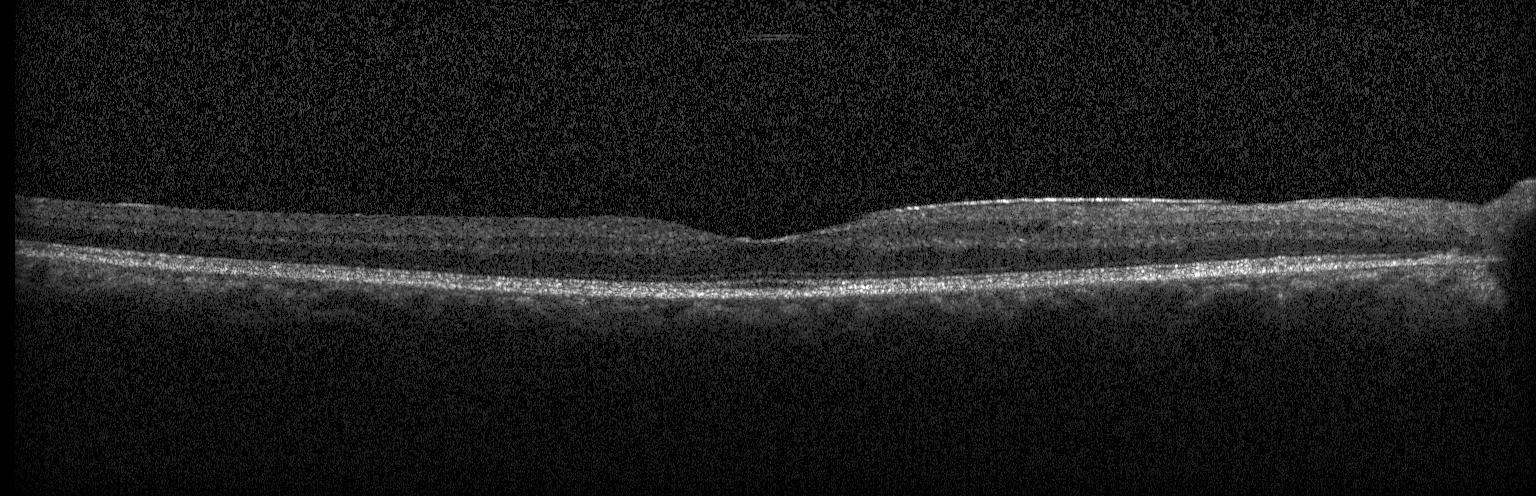 Retinal OCT B-scan; acquired on a Heidelberg Spectralis — Finding: no CNV, DME, or drusen.